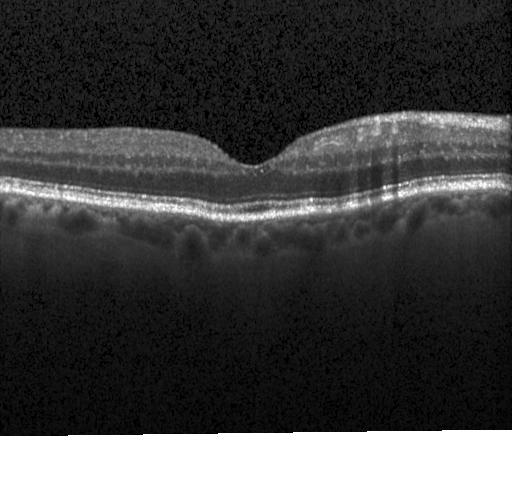

Retinal OCT B-scan. Assessment: no evidence of choroidal neovascularization, diabetic macular edema, or drusen.